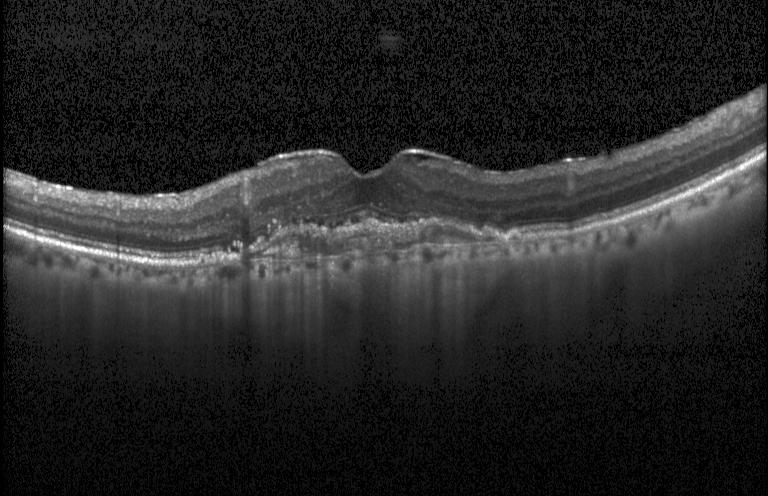

OCT line scan
Dx: a choroidal neovascular membrane.